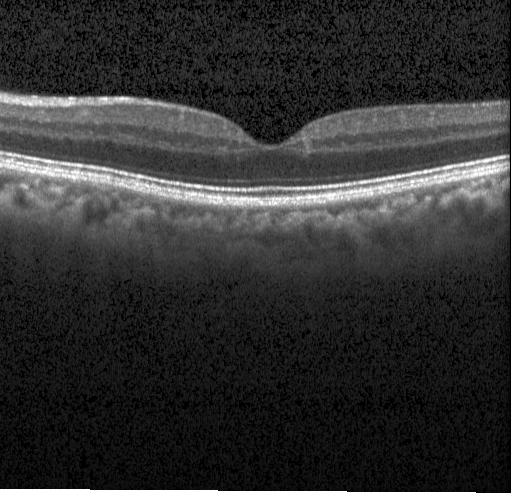

Optical coherence tomography scan; spectral-domain OCT. OCT finding: no choroidal neovascularization, no diabetic macular edema, and no drusen.